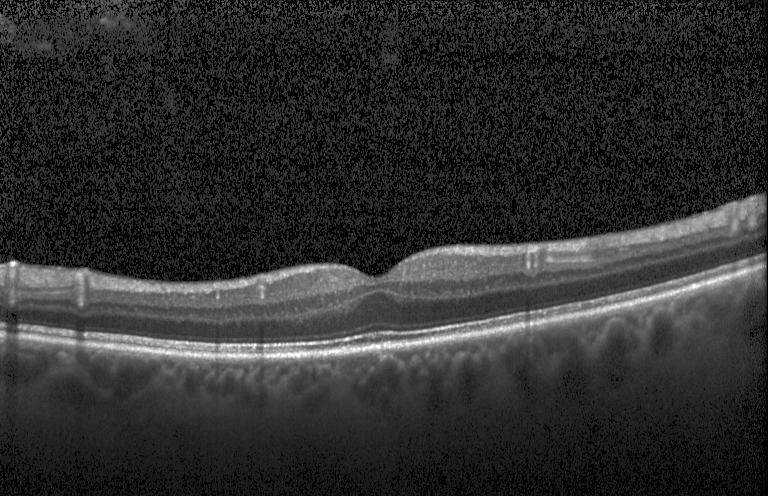
Diagnosis: no choroidal neovascularization, diabetic macular edema, or drusen.